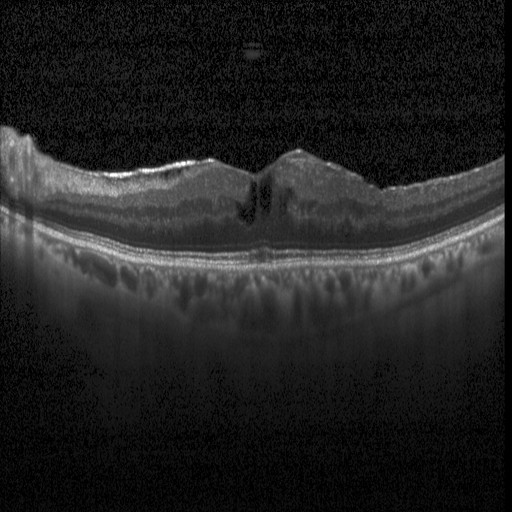
Retinal OCT cross-section. Horizontal scan through the fovea. Instrument: Heidelberg Spectralis. Spectral-domain OCT
Dx: DME.